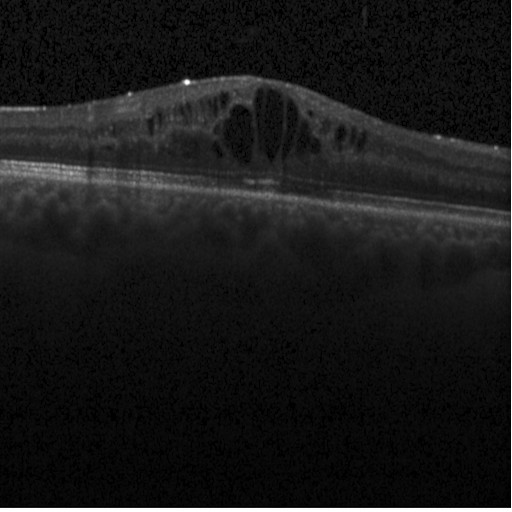
OCT B-scan; acquired on a Heidelberg Spectralis. Diagnosis: DME.